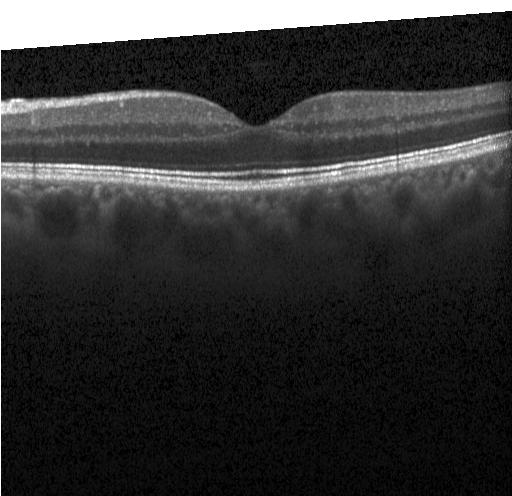

Neither CNV, DME, nor drusen.